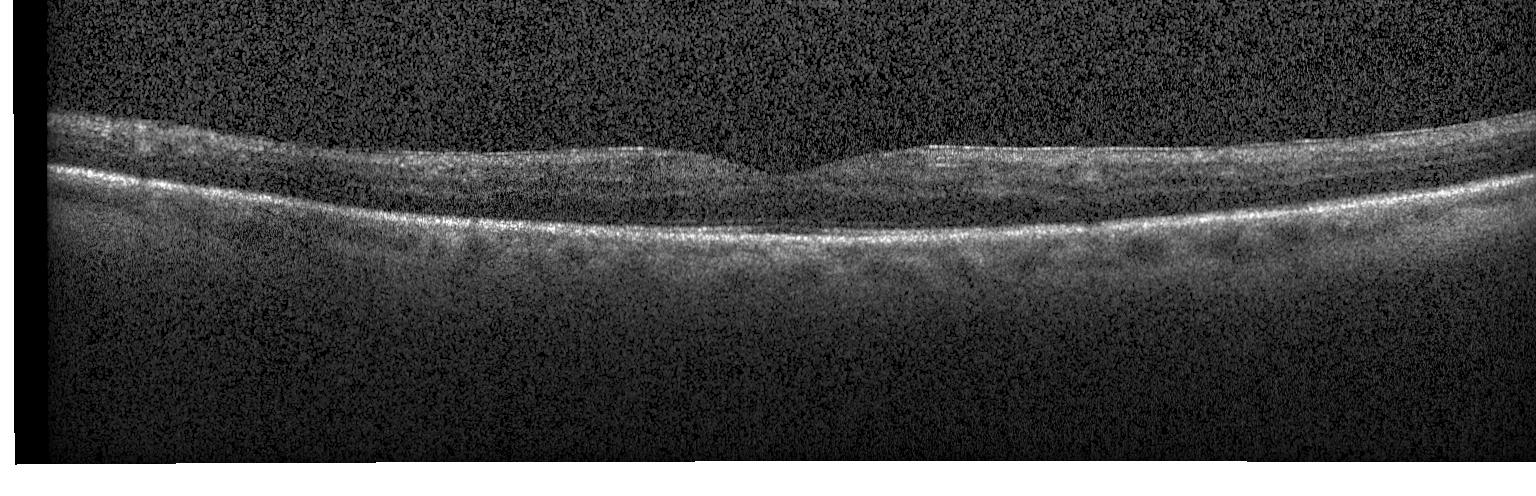 Optical coherence tomography B-scan · macular scan · spectral-domain optical coherence tomography · instrument: Heidelberg Spectralis.
No CNV, DME, or drusen.